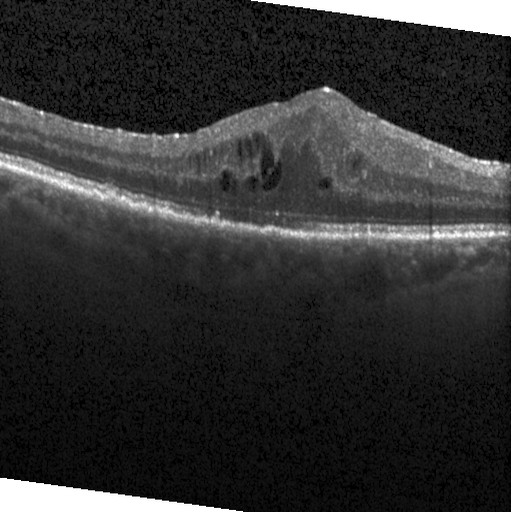
Horizontal scan through the fovea, OCT line scan.
Diabetic macular edema.